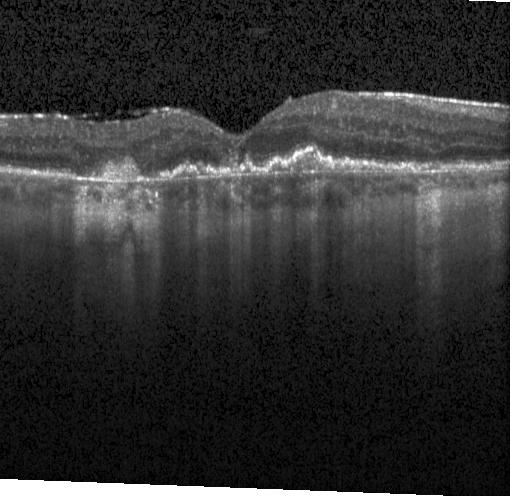

Retinal OCT cross-section showing a choroidal neovascular membrane.